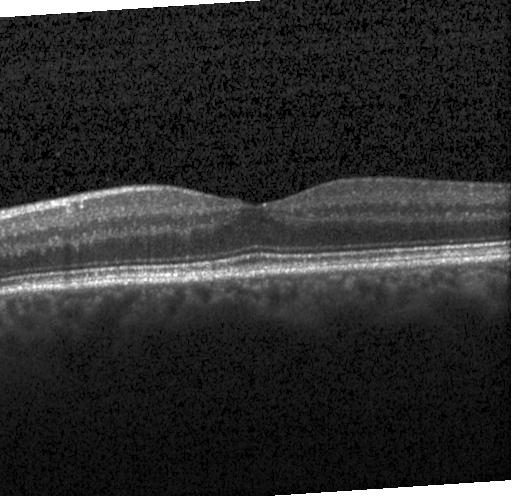
Diagnosis: no CNV, no DME, and no drusen.